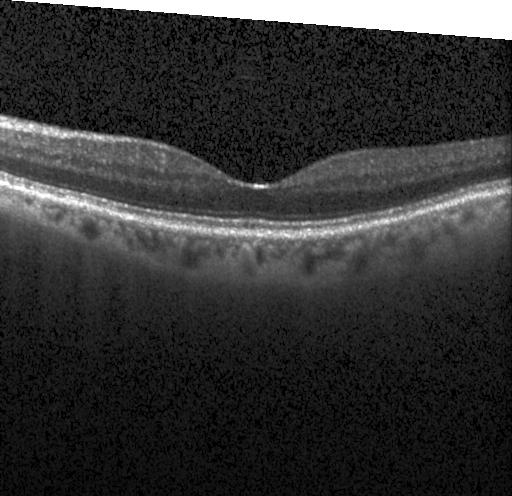
Impression: no evidence of choroidal neovascularization, diabetic macular edema, or drusen.